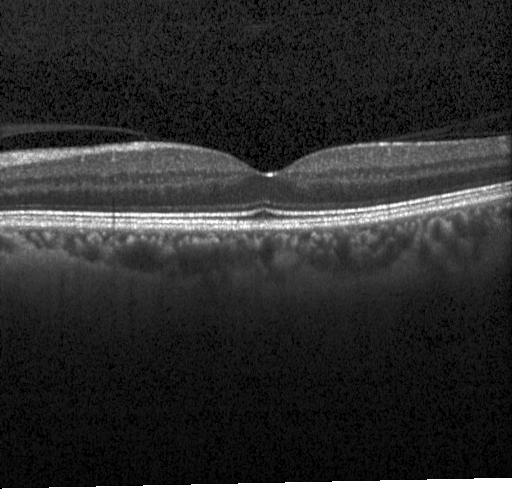
Optical coherence tomography scan
Dx: no choroidal neovascularization, diabetic macular edema, or drusen.